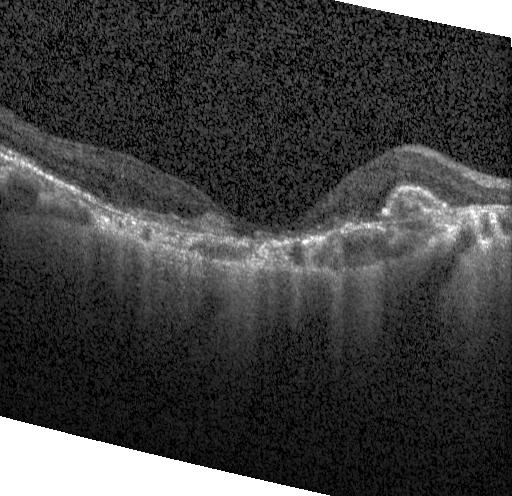 Heidelberg Spectralis; retinal OCT B-scan — The scan shows a choroidal neovascular membrane.